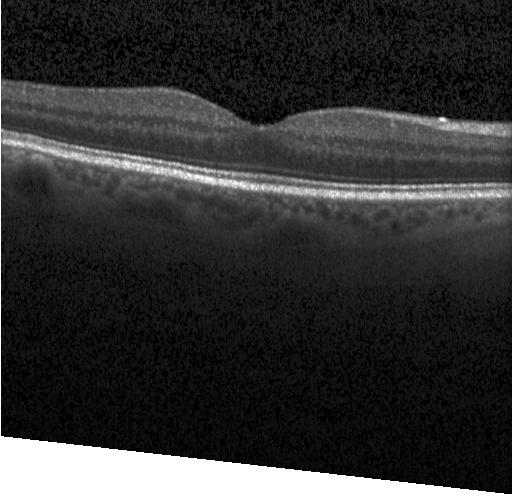

Spectral-domain OCT, macular scan, acquired on a Heidelberg Spectralis, optical coherence tomography B-scan.
Impression: no CNV, no DME, and no drusen.